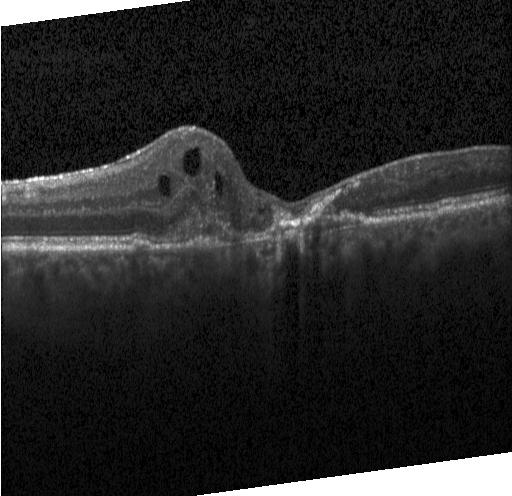

Impression: choroidal neovascularization (CNV).